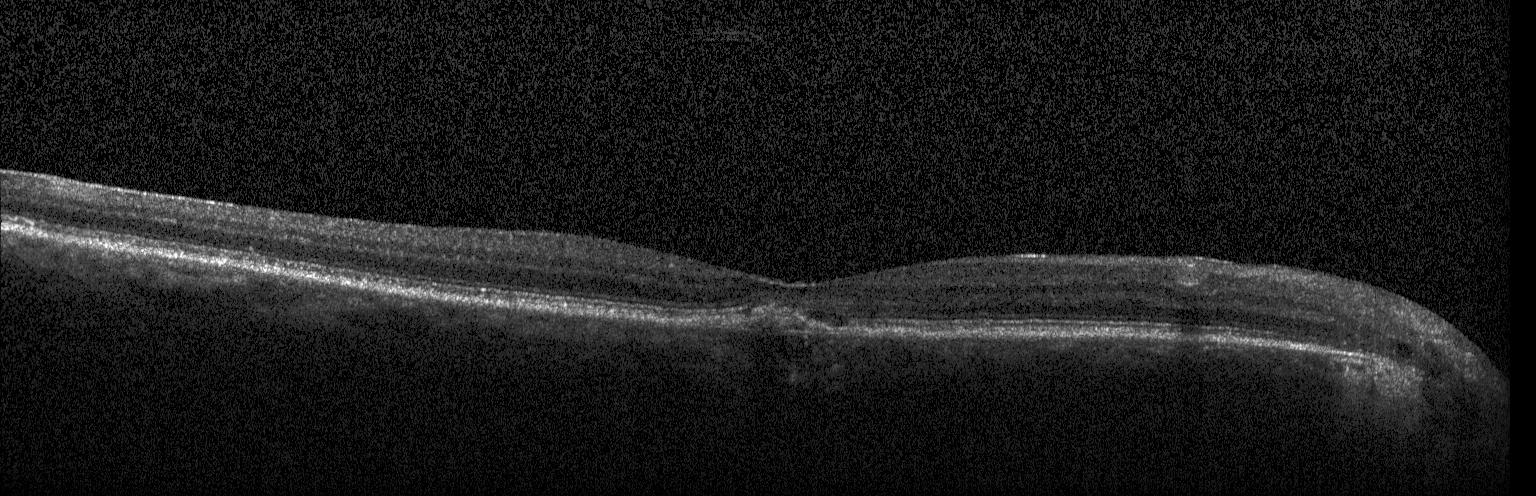
Impression: choroidal neovascularization.